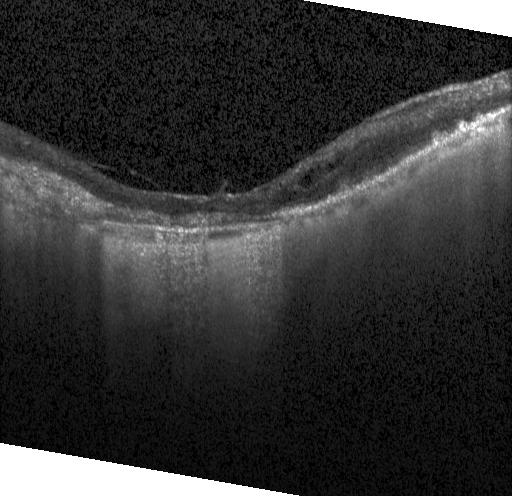
Retinal OCT B-scan. Diagnosis: a choroidal neovascular membrane.